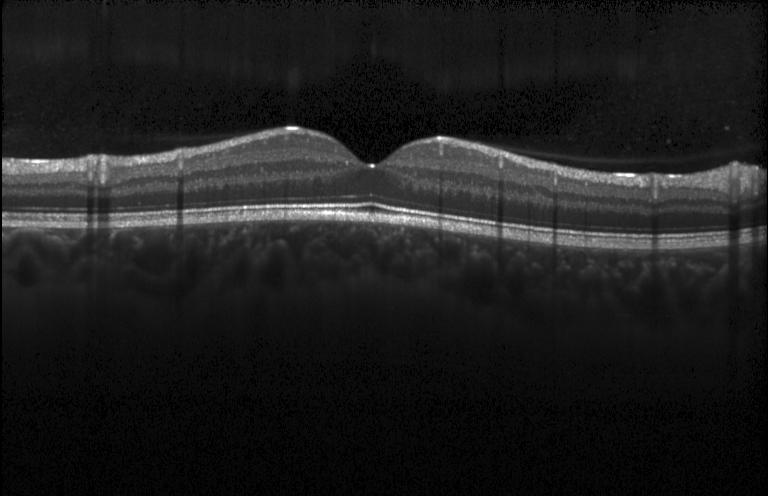 Optical coherence tomography scan — Finding: no evidence of CNV, DME, or drusen.